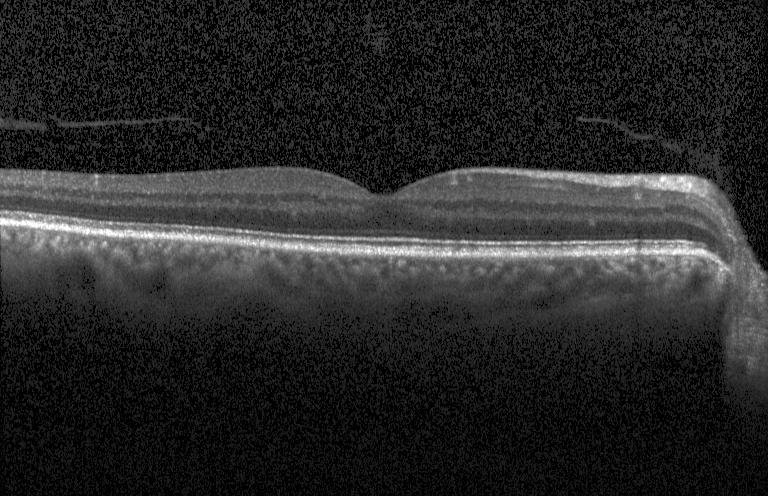 Fovea-centered; OCT line scan
Finding: no evidence of choroidal neovascularization, diabetic macular edema, or drusen.